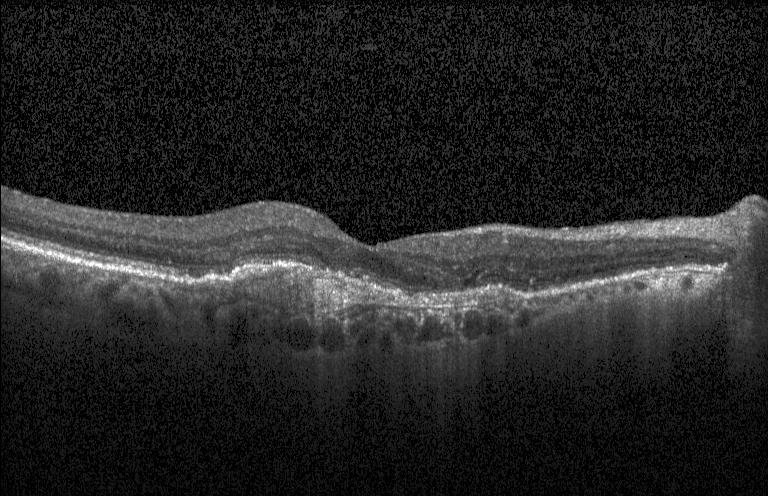
Heidelberg Spectralis OCT system. OCT B-scan
Finding: choroidal neovascularization (CNV).